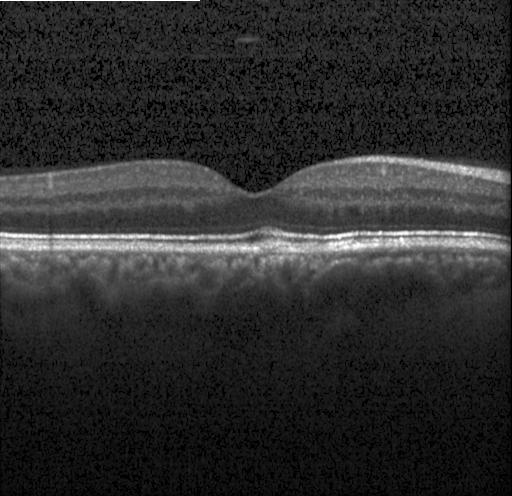 Dx: no evidence of CNV, DME, or drusen.